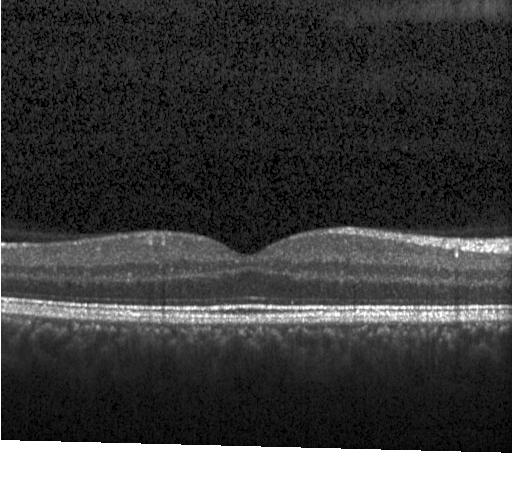

Through the macula. Optical coherence tomography B-scan
Impression: no evidence of CNV, DME, or drusen.